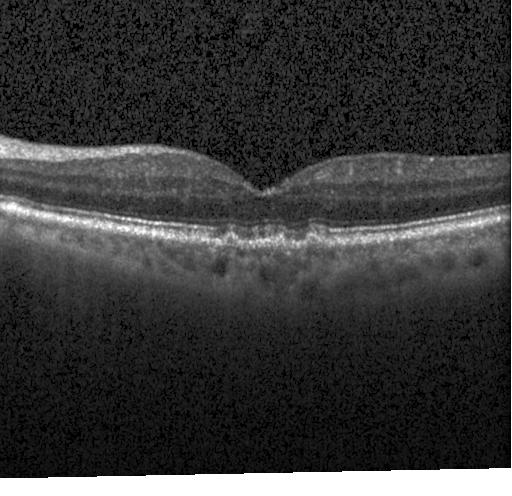
Retinal OCT cross-section, horizontal scan through the fovea, spectral-domain OCT — Finding: multiple drusen.